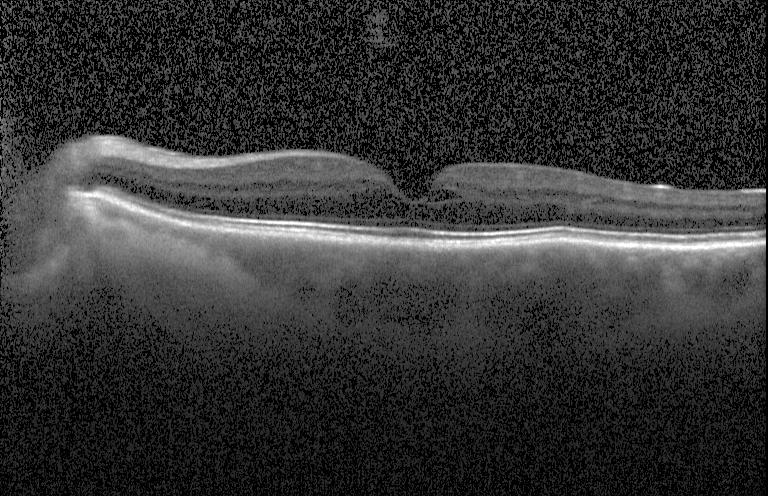
Optical coherence tomography scan
Diabetic macular edema.